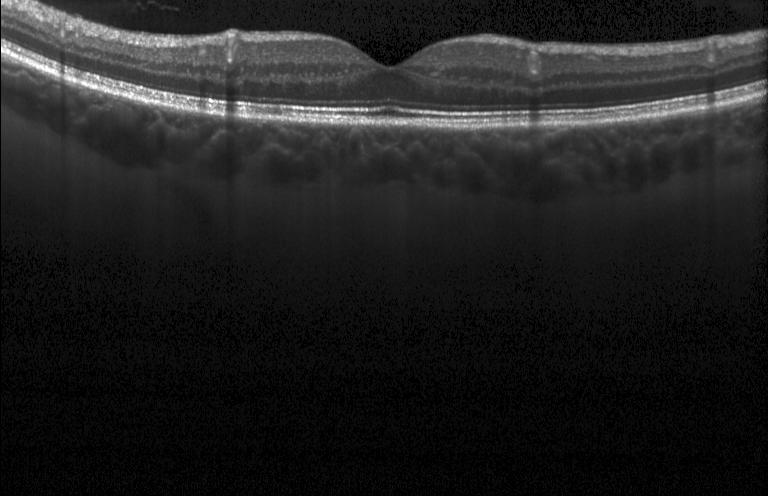

SD-OCT · OCT B-scan · Heidelberg Spectralis OCT system · fovea-centered.
This B-scan demonstrates no evidence of CNV, DME, or drusen.